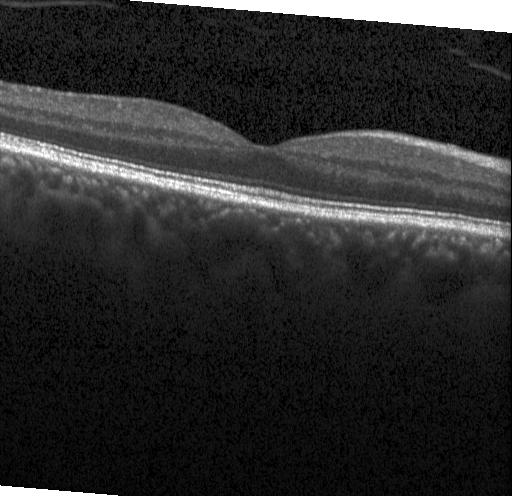

Acquired on a Heidelberg Spectralis, OCT line scan.
No choroidal neovascularization, no diabetic macular edema, and no drusen.